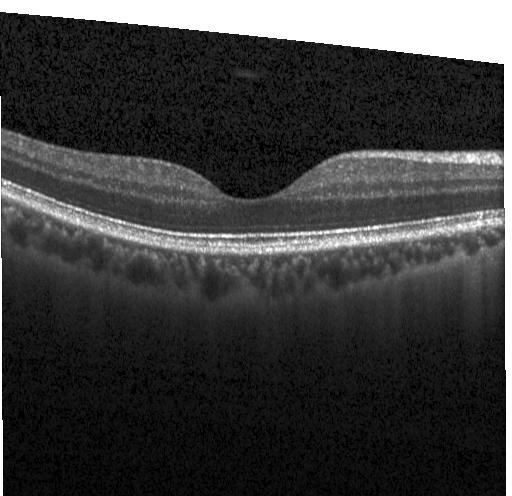

This B-scan demonstrates no choroidal neovascularization, diabetic macular edema, or drusen.